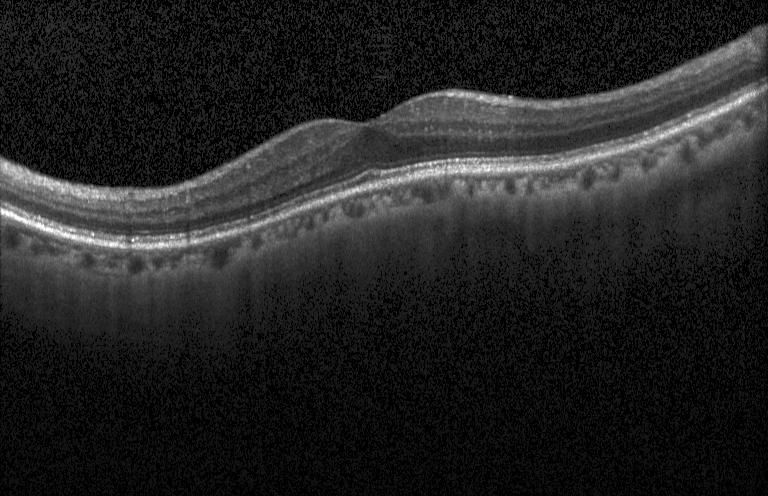
Diagnosis: no CNV, DME, or drusen.